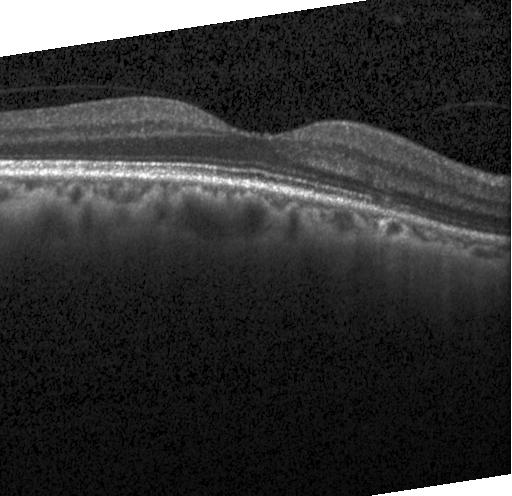 Retinal OCT B-scan · macular scan · Heidelberg Spectralis · SD-OCT — Impression: no choroidal neovascularization, diabetic macular edema, or drusen.